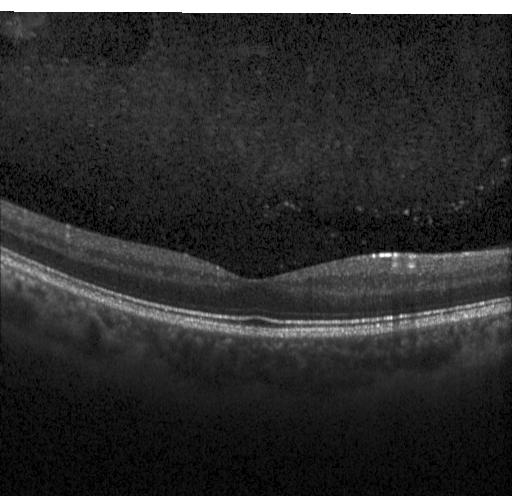
Macular scan; retinal OCT cross-section; Heidelberg Spectralis OCT system — Dx: no choroidal neovascularization, no diabetic macular edema, and no drusen.